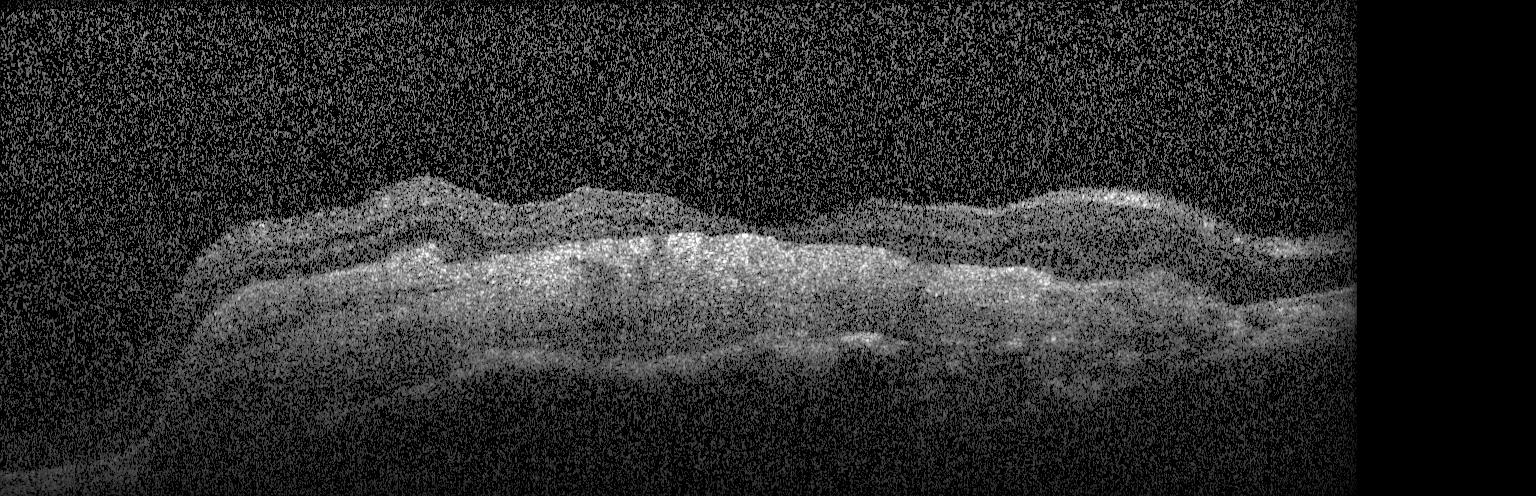

OCT finding: a choroidal neovascular membrane.